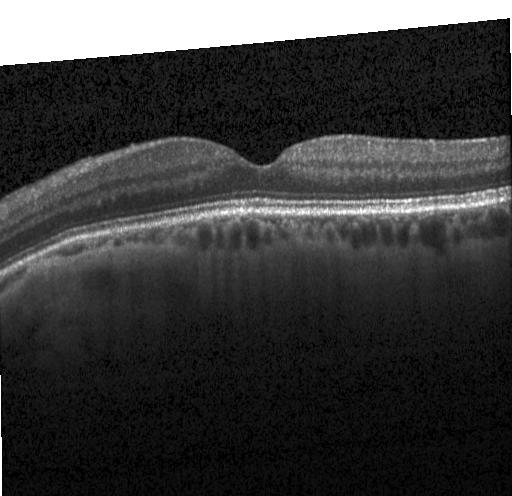 The scan shows no choroidal neovascularization, diabetic macular edema, or drusen.